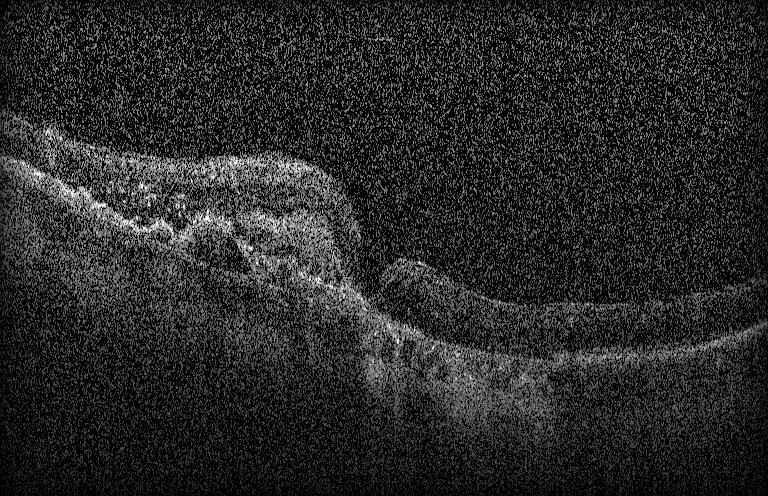
Optical coherence tomography B-scan — Assessment: choroidal neovascularization (CNV).